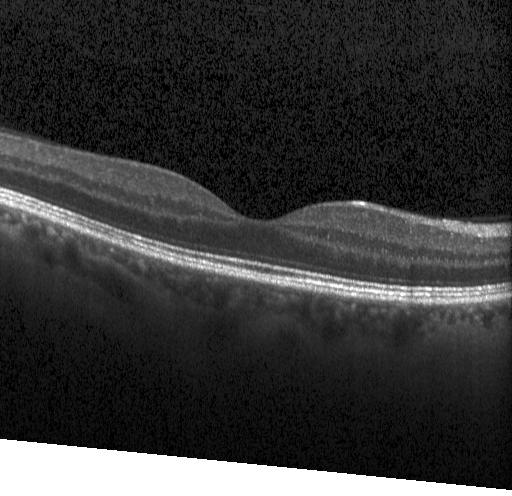

Spectral-domain OCT, fovea-centered, OCT B-scan. Diagnosis: no evidence of choroidal neovascularization, diabetic macular edema, or drusen.